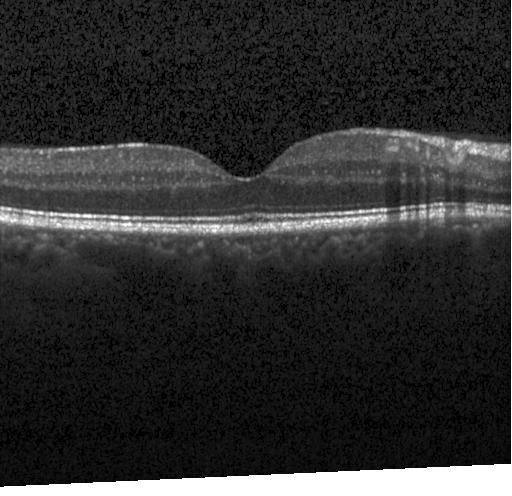
Horizontal scan through the fovea. OCT line scan. Heidelberg Spectralis OCT system
Impression: no evidence of choroidal neovascularization, diabetic macular edema, or drusen.